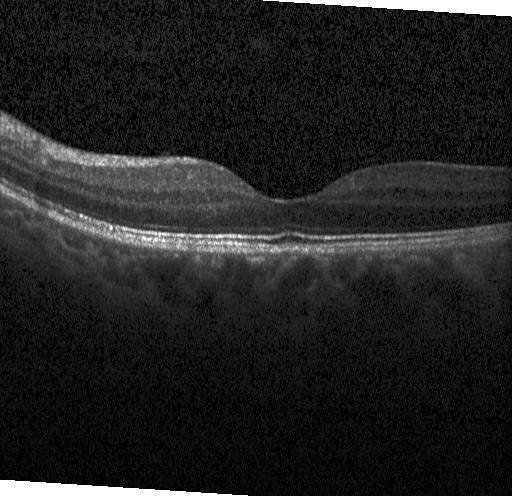

Macular OCT: no choroidal neovascularization, no diabetic macular edema, and no drusen.